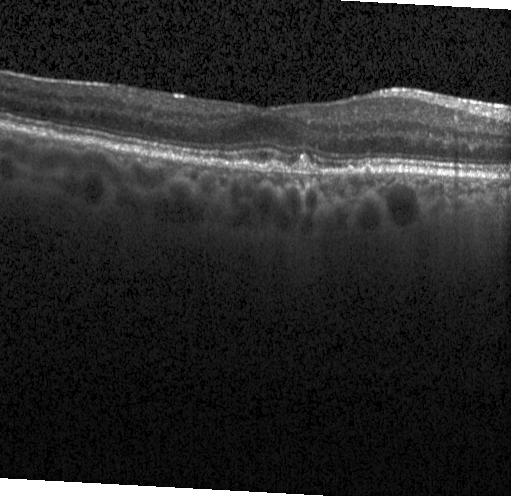 Retinal OCT B-scan, Heidelberg Spectralis OCT system, through the macula
OCT finding: drusen.